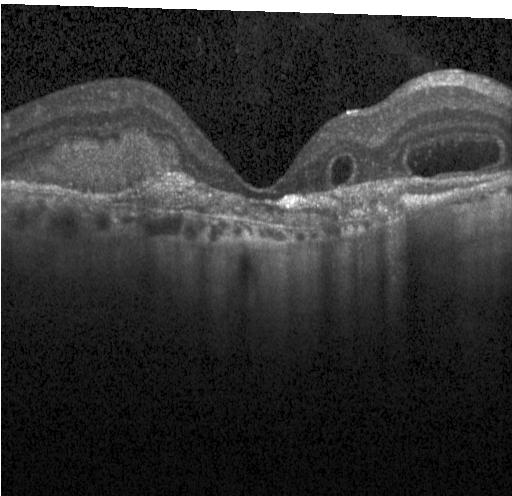
Impression: CNV.